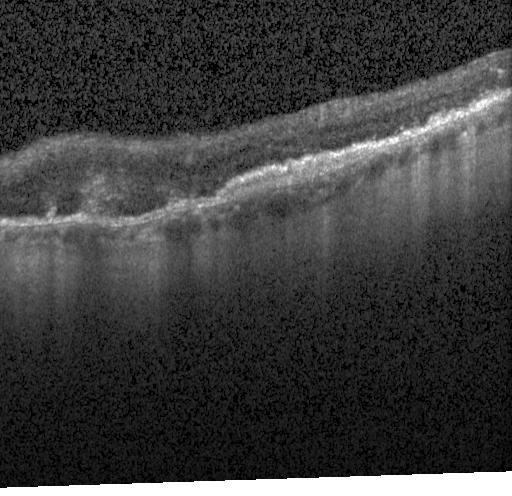 Diagnosis: a choroidal neovascular membrane.